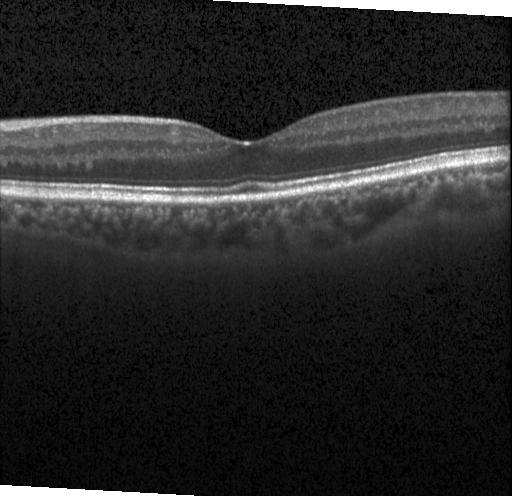 Optical coherence tomography B-scan. Spectral-domain optical coherence tomography. Heidelberg Spectralis. The scan shows no choroidal neovascularization, diabetic macular edema, or drusen.